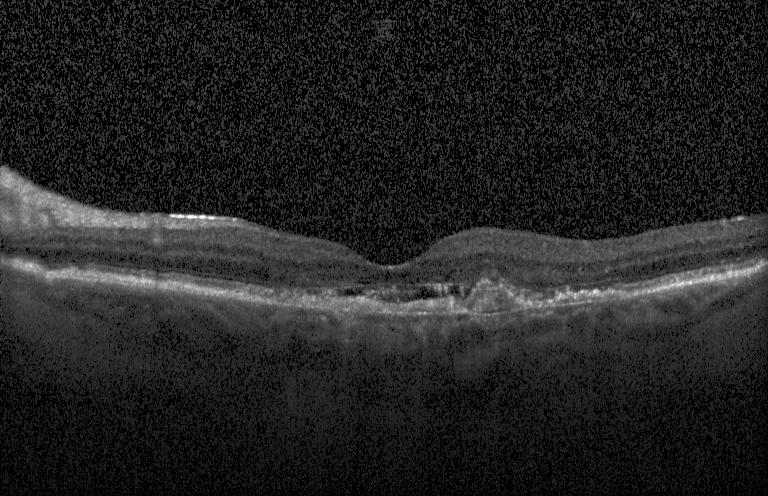

Impression: CNV.